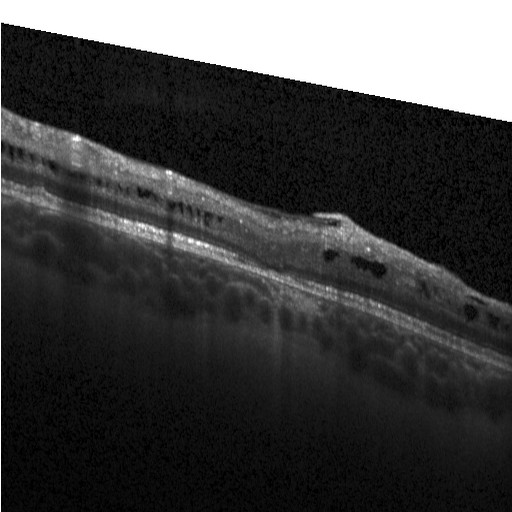 Diabetic macular edema.